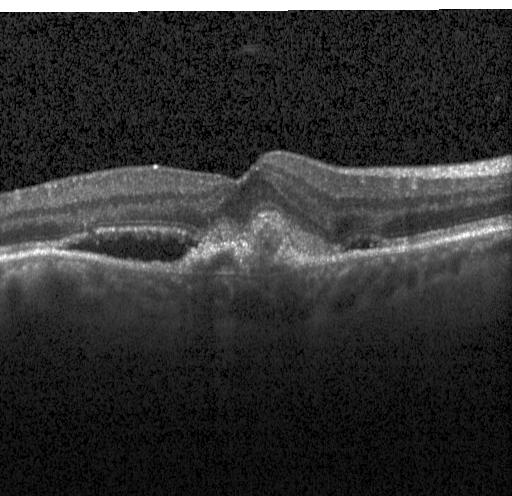
Macular OCT: CNV.